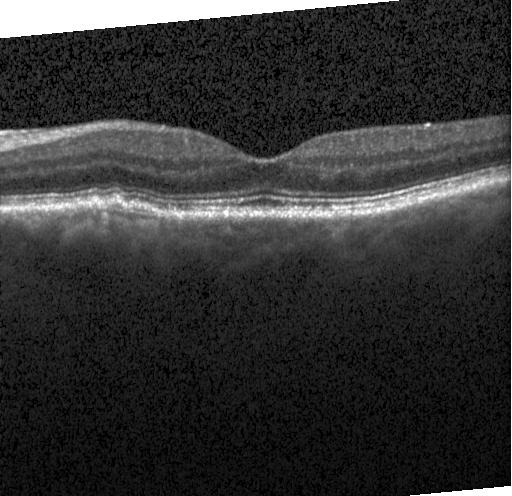
Horizontal scan through the fovea, Heidelberg Spectralis, retinal OCT cross-section.
Finding: drusen.